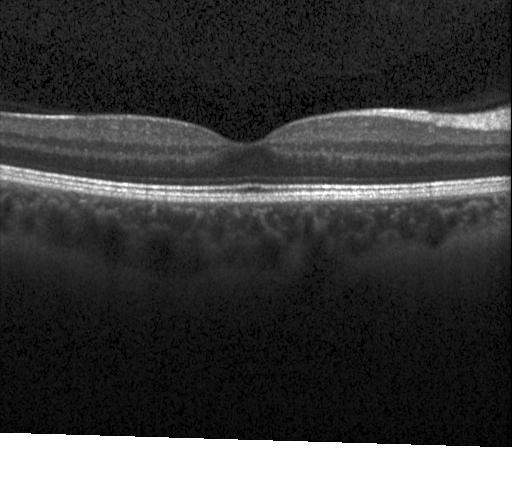

Retinal OCT cross-section · fovea-centered
Diagnosis: no evidence of choroidal neovascularization, diabetic macular edema, or drusen.